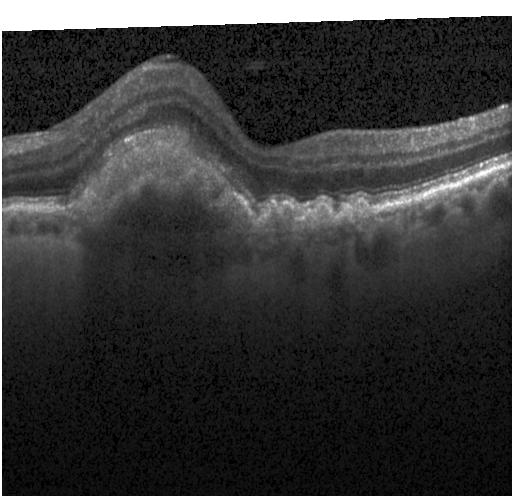
Spectral-domain OCT. Macular scan. Optical coherence tomography B-scan. CNV.